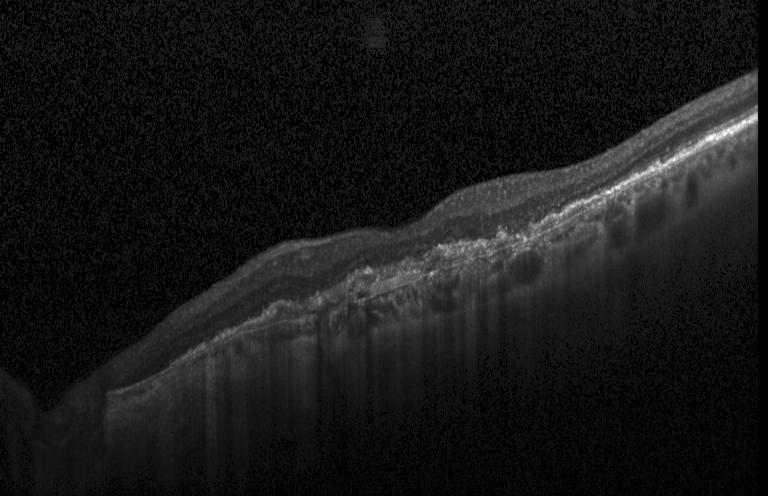

OCT line scan.
Dx: choroidal neovascularization.